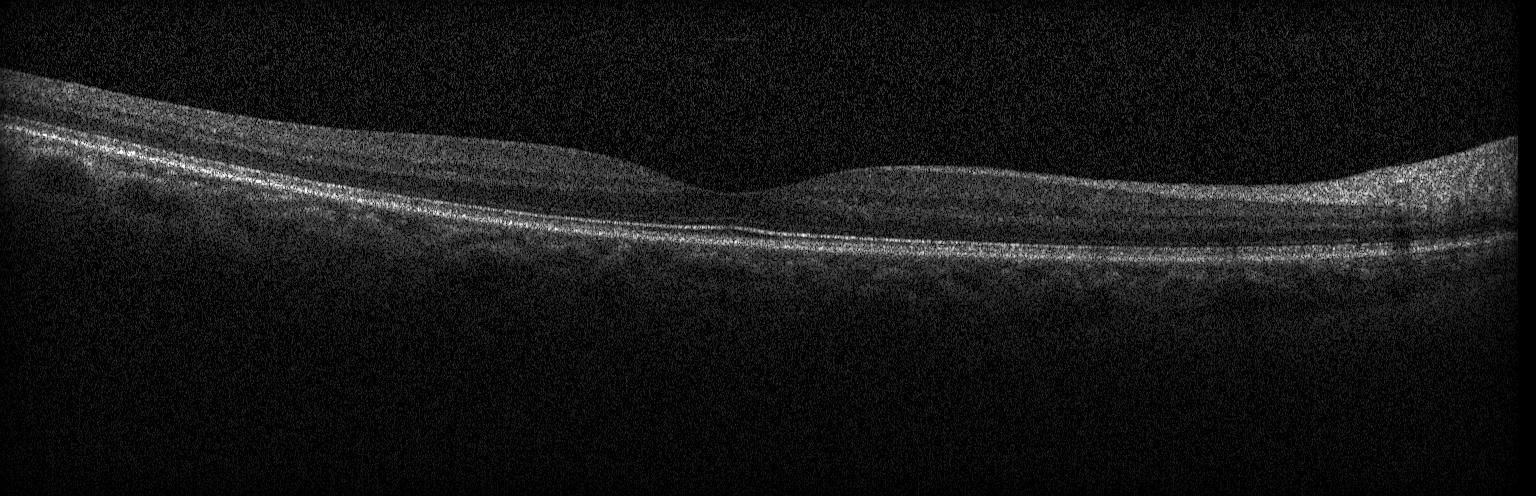 OCT scan showing no choroidal neovascularization, no diabetic macular edema, and no drusen.